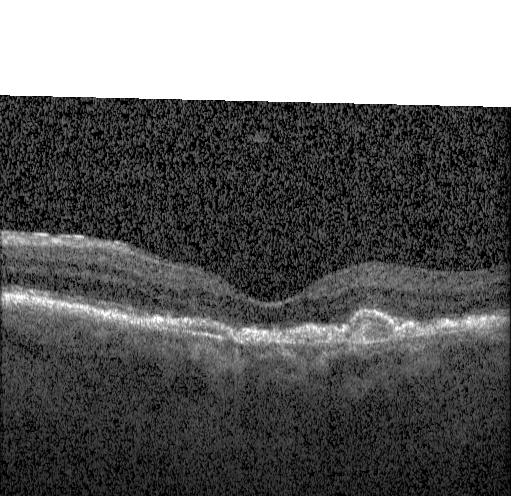

Diagnosis: a choroidal neovascular membrane.